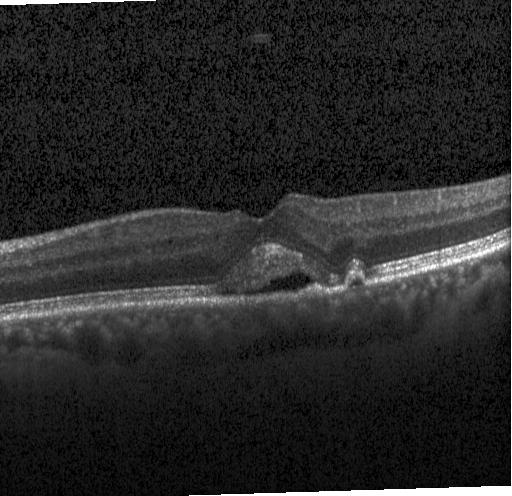
OCT B-scan, fovea-centered. Finding: a choroidal neovascular membrane.